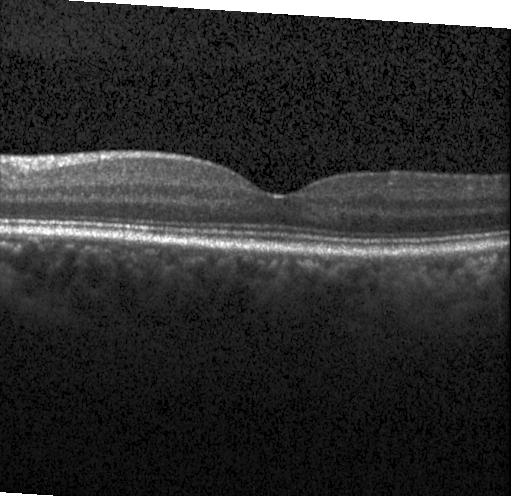

Instrument: Heidelberg Spectralis, optical coherence tomography scan, horizontal scan through the fovea, spectral-domain OCT — Macular OCT: no evidence of choroidal neovascularization, diabetic macular edema, or drusen.